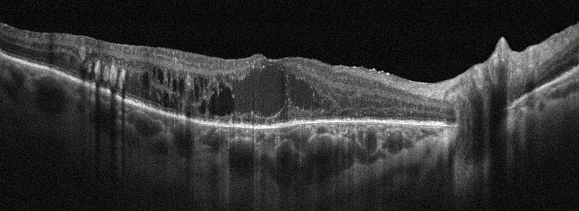
Impression: diabetic macular edema.